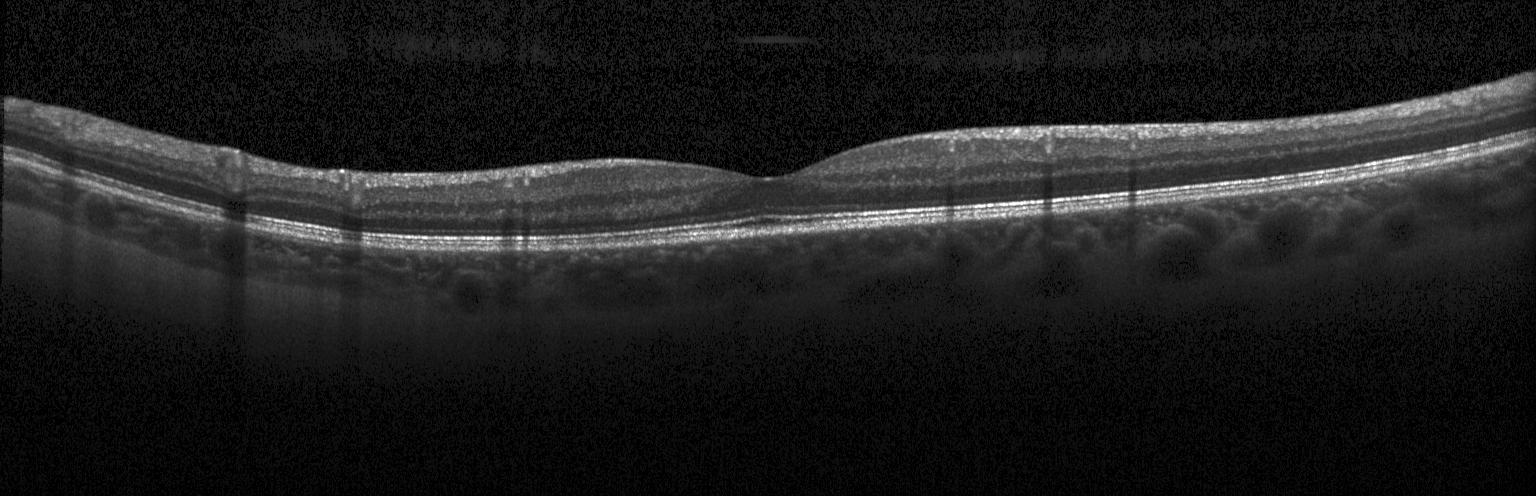

Retinal OCT cross-section; acquired on a Heidelberg Spectralis. The scan shows neither CNV, DME, nor drusen.